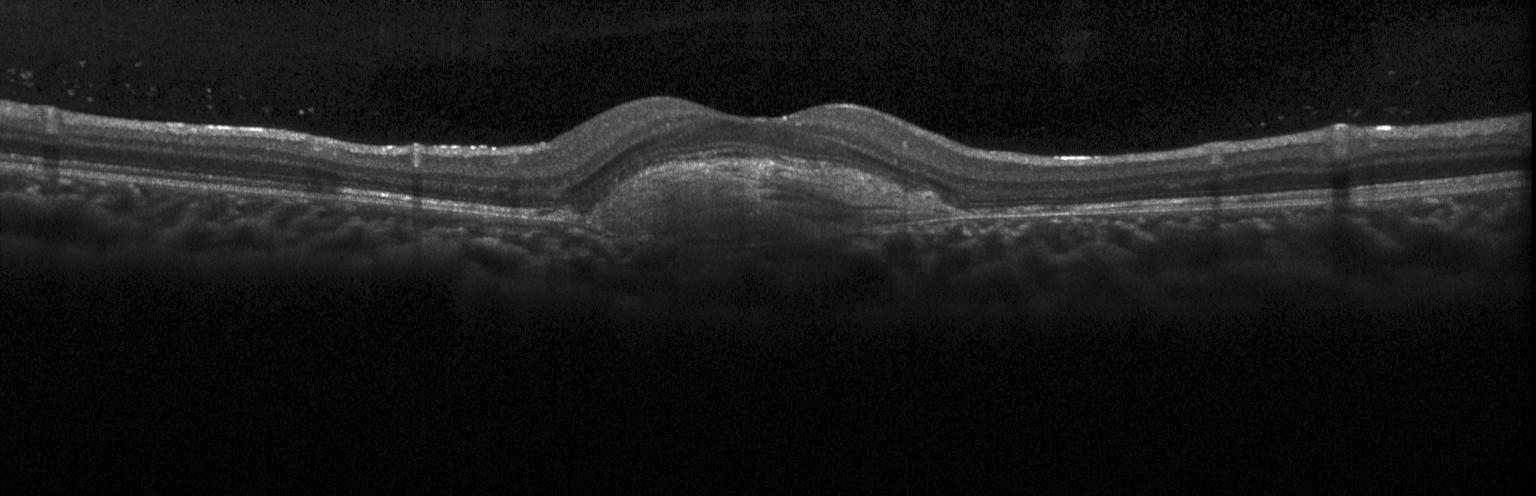

Macular OCT: a choroidal neovascular membrane.